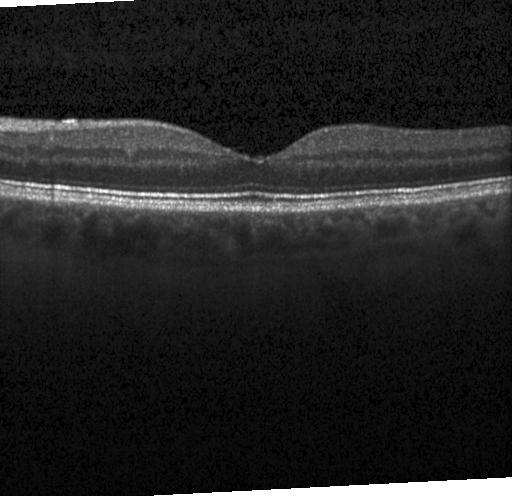
Retinal OCT B-scan. Spectral-domain optical coherence tomography — This B-scan demonstrates no choroidal neovascularization, diabetic macular edema, or drusen.